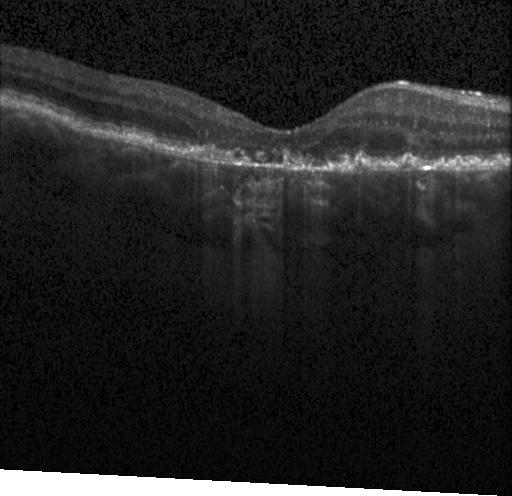
Finding: CNV.